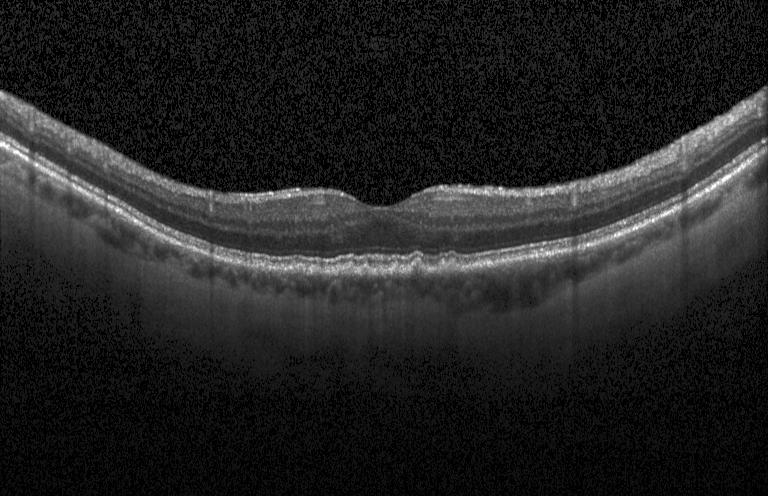 Retinal OCT B-scan
The scan shows sub-RPE drusenoid deposits.